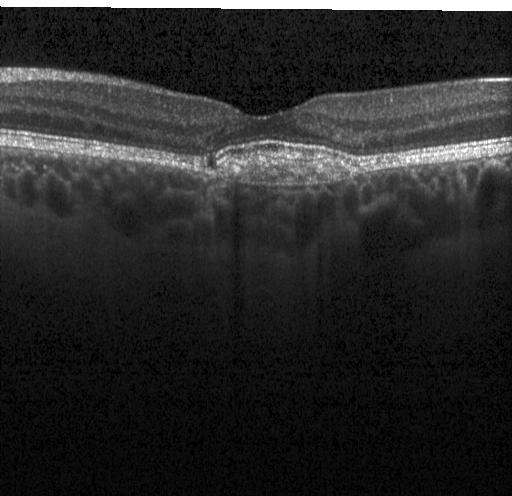 This B-scan demonstrates a choroidal neovascular membrane.